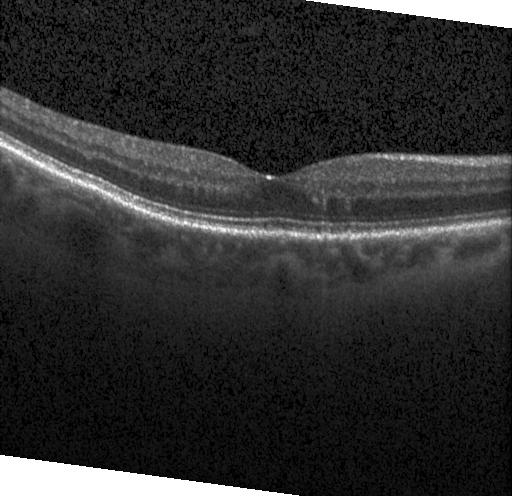

Macular OCT: no CNV, DME, or drusen.